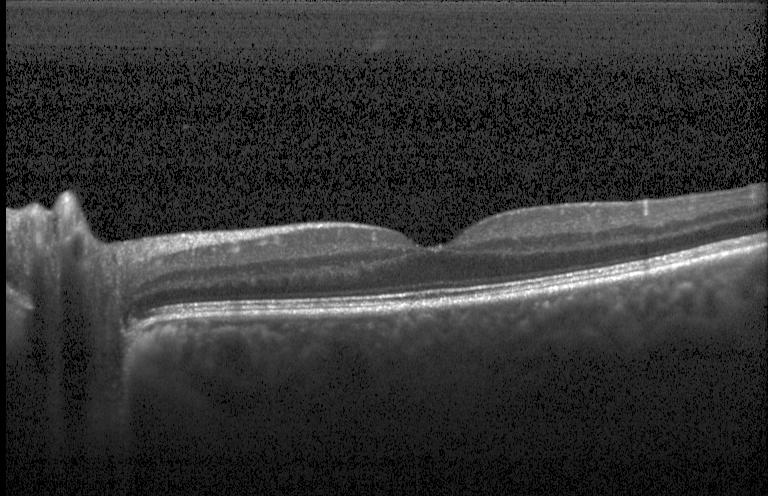

Impression: no choroidal neovascularization, no diabetic macular edema, and no drusen.